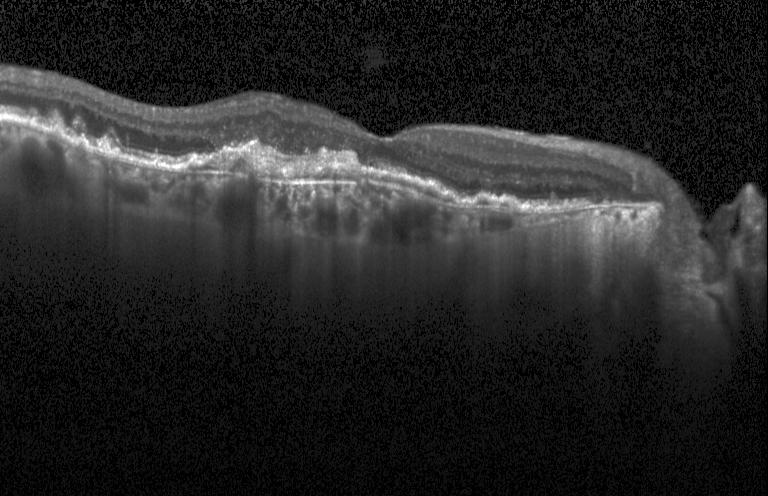 Optical coherence tomography scan. Choroidal neovascularization (CNV).